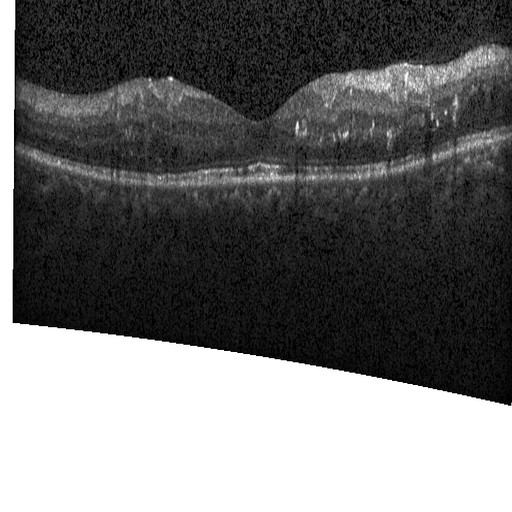

This B-scan demonstrates diabetic macular edema.